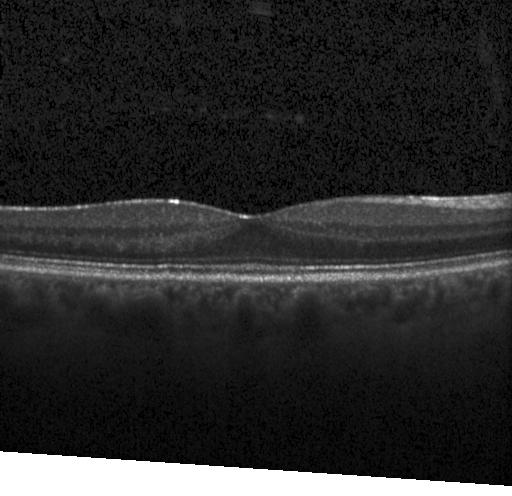

SD-OCT. OCT B-scan. Heidelberg Spectralis
No evidence of CNV, DME, or drusen.